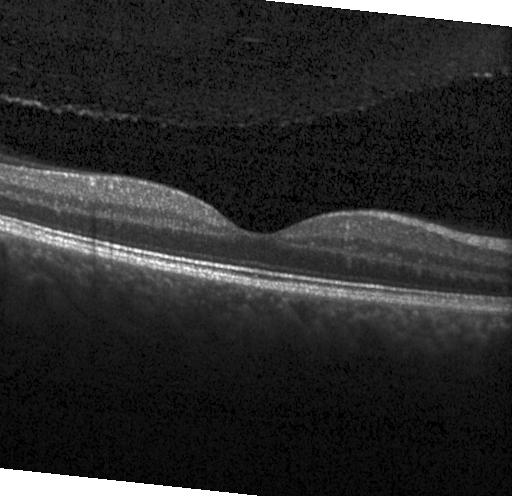
Retinal OCT B-scan.
Impression: no CNV, no DME, and no drusen.